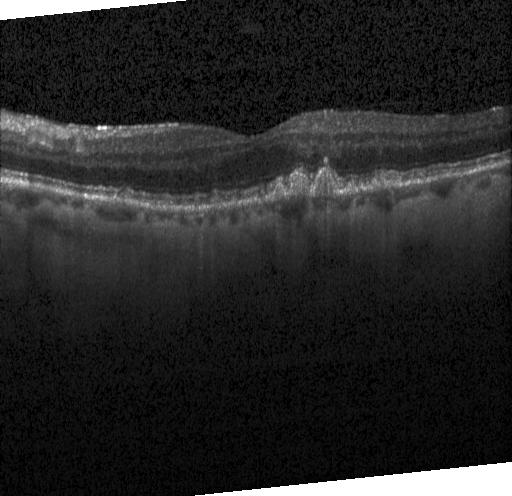 OCT line scan.
OCT finding: sub-RPE drusenoid deposits.